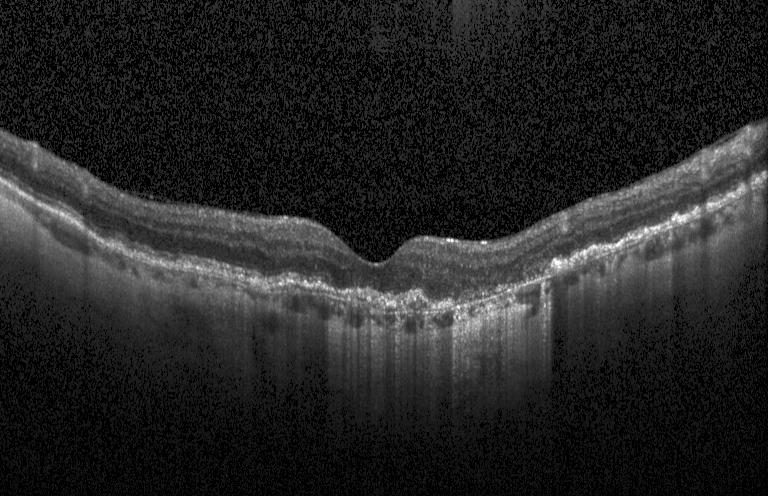

Macular OCT: a choroidal neovascular membrane.